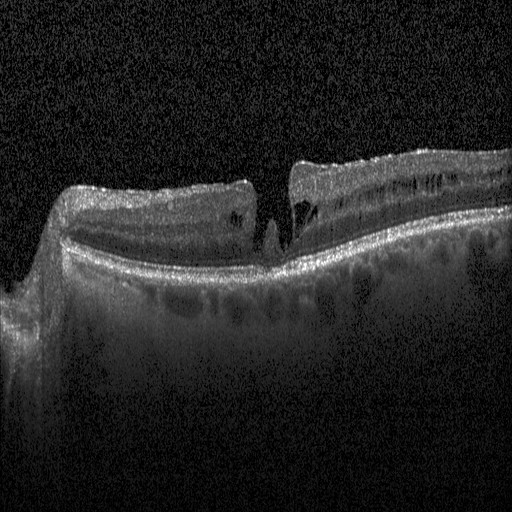

Fovea-centered, retinal OCT cross-section, spectral-domain OCT
Diagnosis: diabetic macular edema (DME).